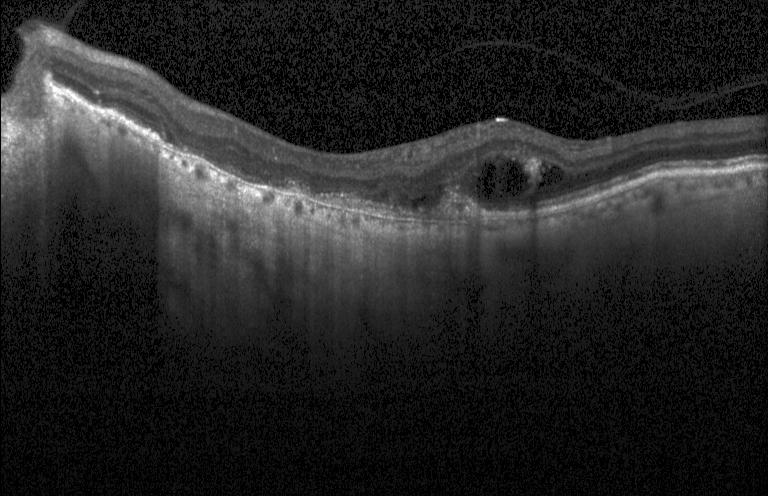
Heidelberg Spectralis; macular scan; OCT B-scan; spectral-domain optical coherence tomography.
Finding: a choroidal neovascular membrane.